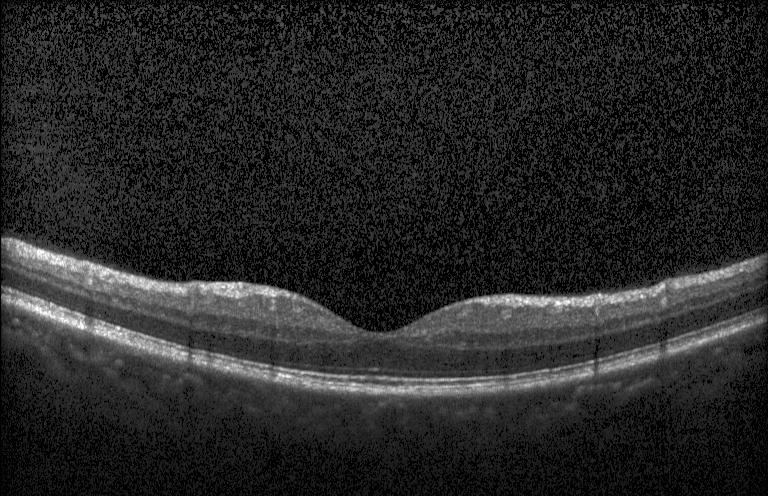 Acquired on a Heidelberg Spectralis, horizontal scan through the fovea, optical coherence tomography B-scan — Finding: no CNV, DME, or drusen.